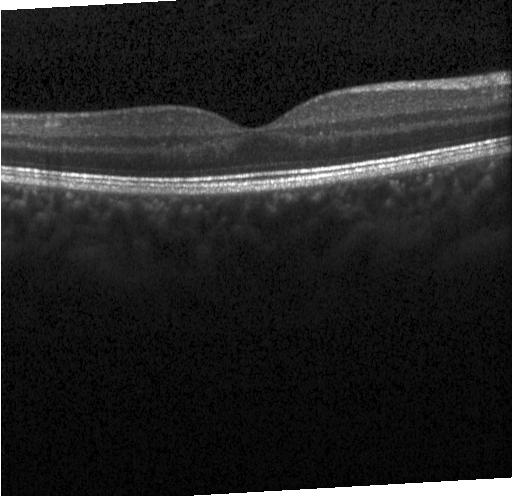 OCT line scan. Spectral-domain OCT
Dx: neither choroidal neovascularization, diabetic macular edema, nor drusen.